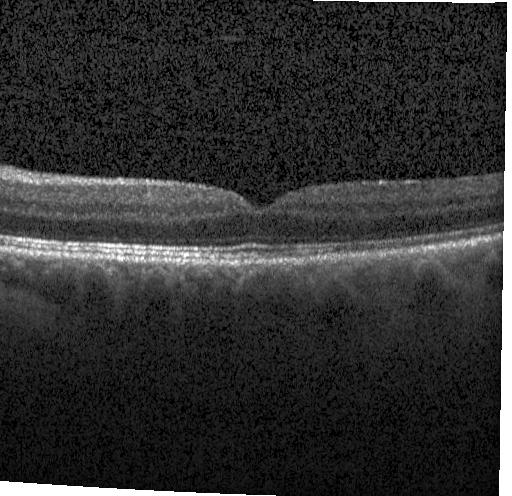 Diagnosis: neither choroidal neovascularization, diabetic macular edema, nor drusen.